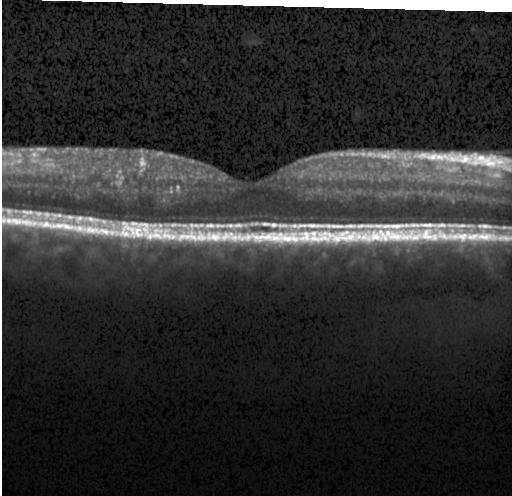
OCT scan showing no evidence of choroidal neovascularization, diabetic macular edema, or drusen.